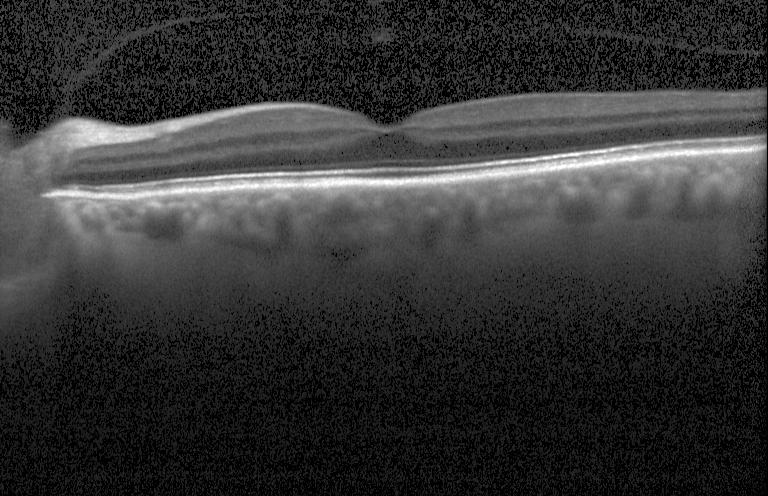

Diagnosis: no evidence of choroidal neovascularization, diabetic macular edema, or drusen.